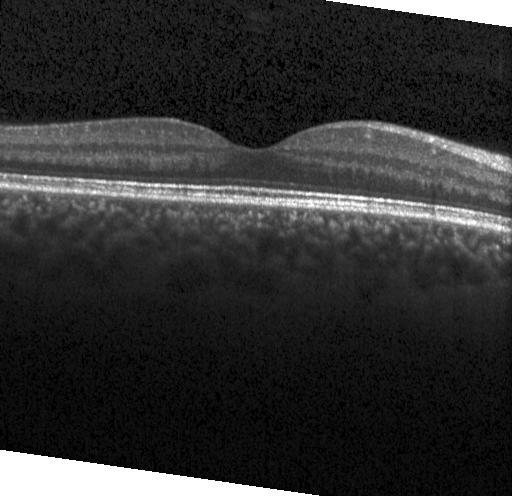 Macular OCT demonstrating no evidence of choroidal neovascularization, diabetic macular edema, or drusen.